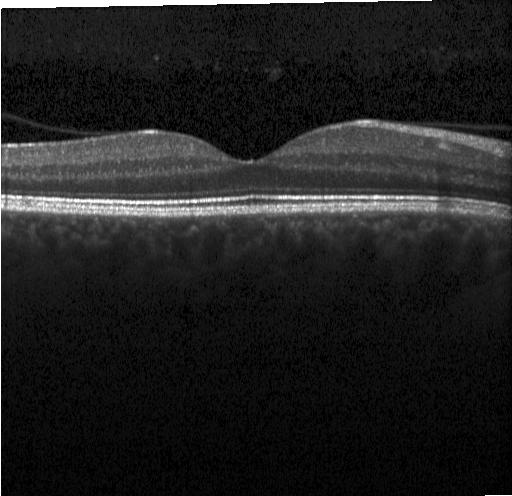
Spectral-domain OCT. Retinal OCT cross-section
Diagnosis: neither CNV, DME, nor drusen.